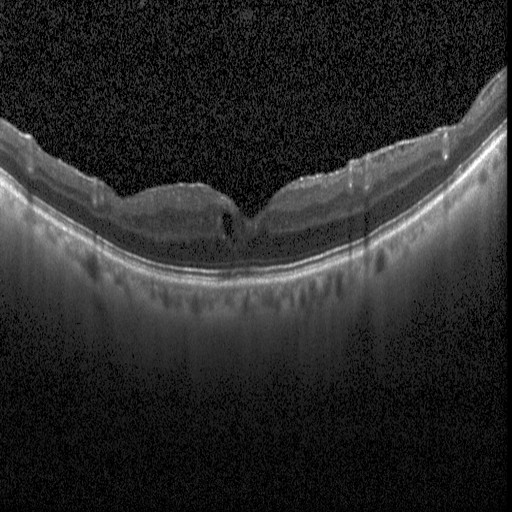

Acquired on a Heidelberg Spectralis; optical coherence tomography B-scan; spectral-domain optical coherence tomography; macular scan — Macular OCT: DME.